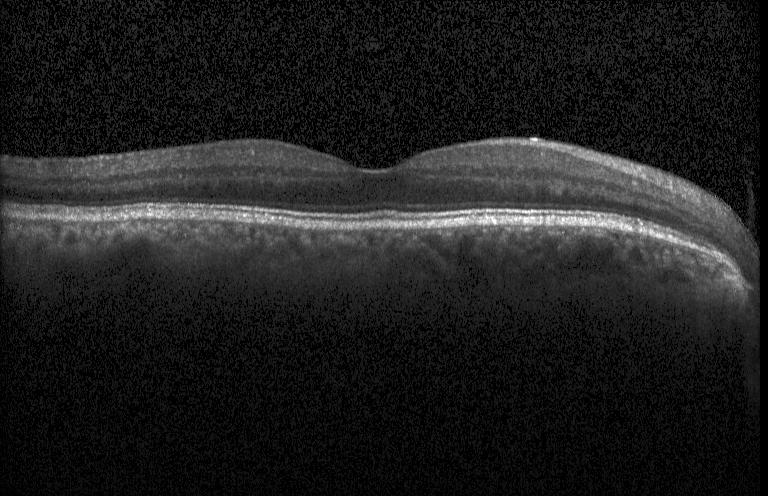 Diagnosis: no CNV, DME, or drusen.